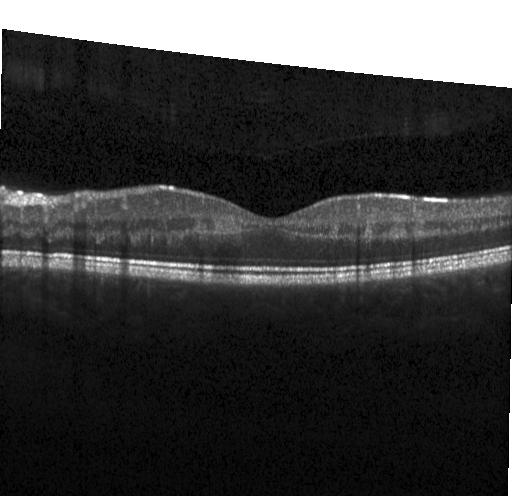 Retinal OCT cross-section showing neither CNV, DME, nor drusen.